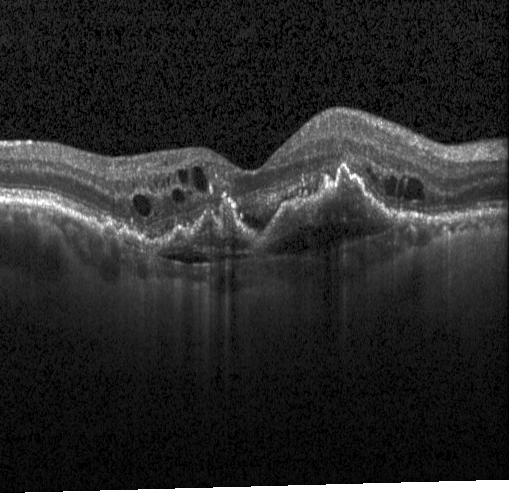 Horizontal scan through the fovea. Acquired on a Heidelberg Spectralis. OCT B-scan.
Finding: choroidal neovascularization (CNV).